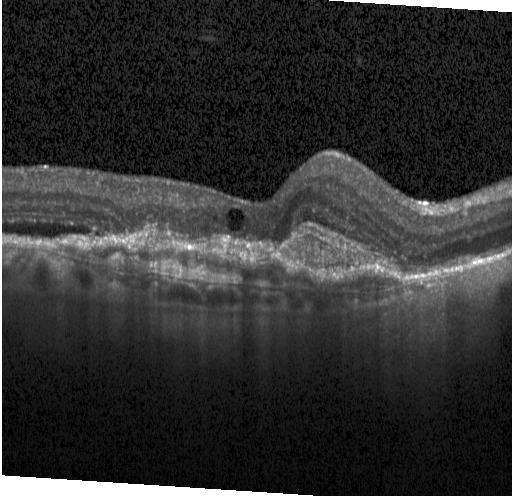 Spectral-domain OCT B-scan: CNV.